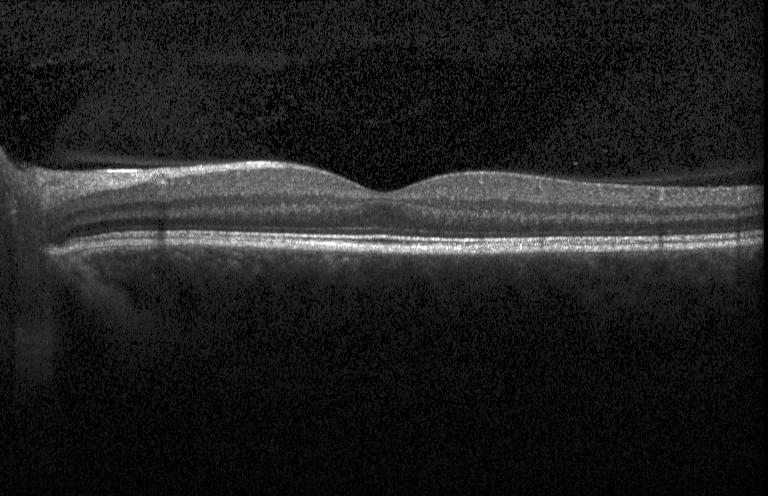
Instrument: Heidelberg Spectralis; spectral-domain optical coherence tomography; horizontal scan through the fovea; OCT line scan.
Impression: no CNV, DME, or drusen.